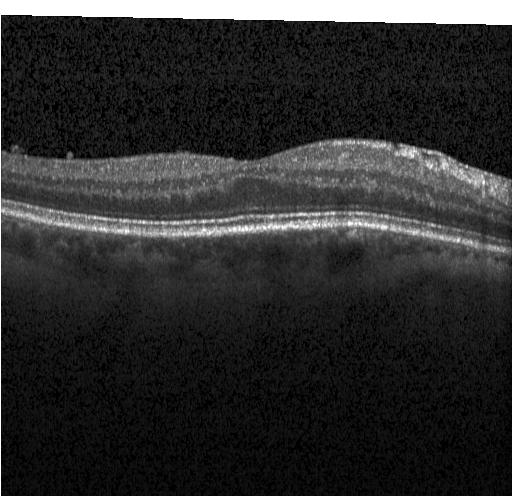
OCT line scan · instrument: Heidelberg Spectralis · centered on the fovea.
No evidence of CNV, DME, or drusen.